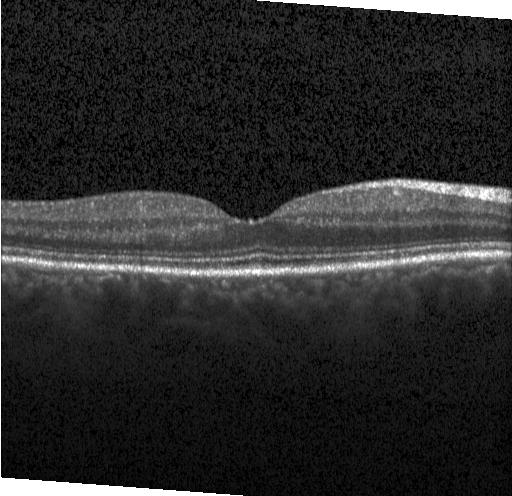

No choroidal neovascularization, no diabetic macular edema, and no drusen.